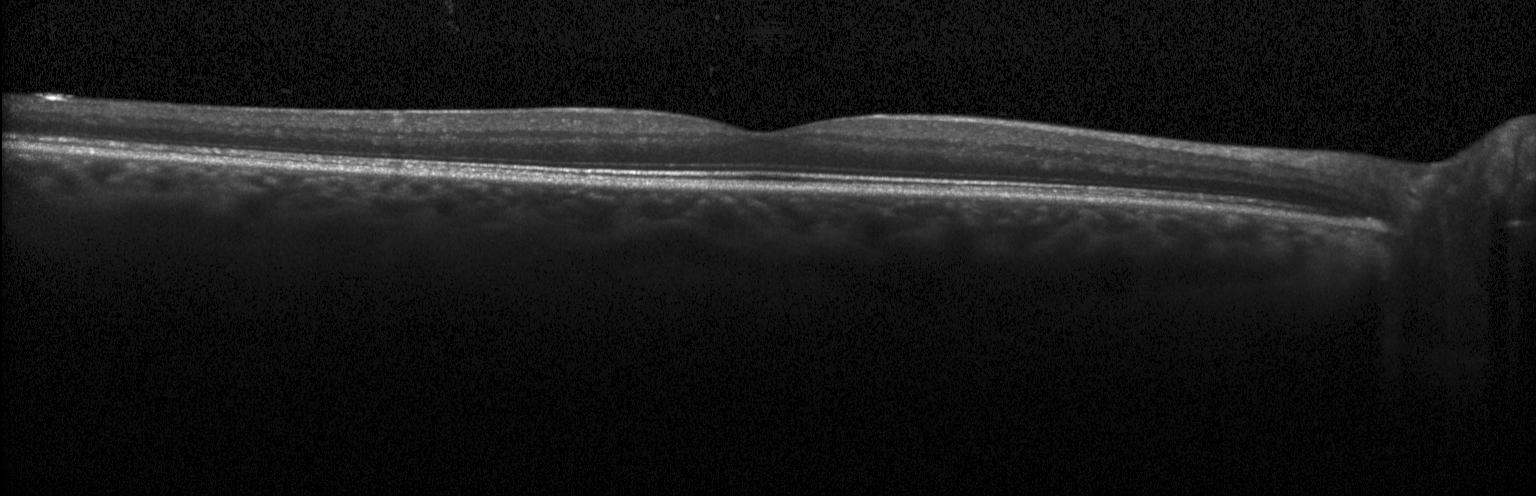
Spectral-domain OCT B-scan: no choroidal neovascularization, no diabetic macular edema, and no drusen.